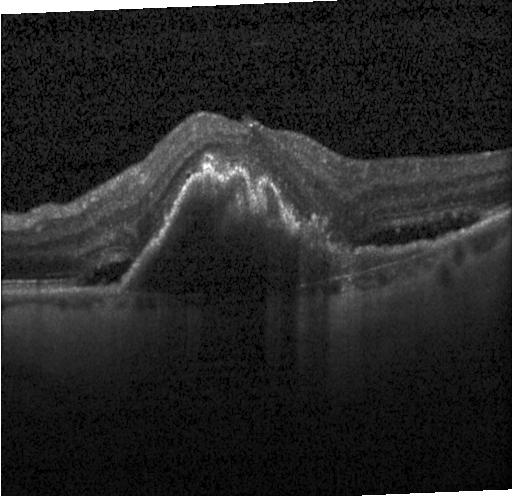
Spectral-domain OCT; acquired on a Heidelberg Spectralis; optical coherence tomography scan.
Diagnosis: a choroidal neovascular membrane.